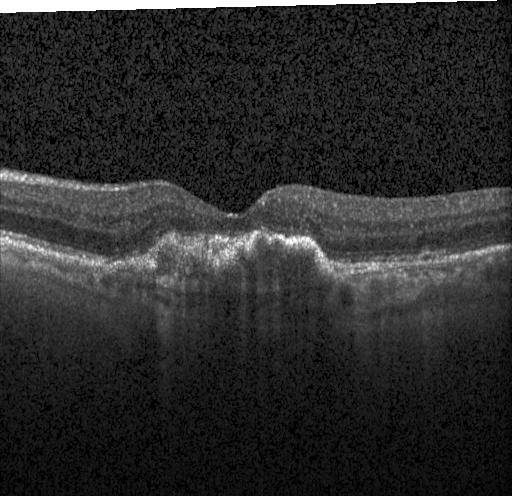
OCT line scan — Macular OCT: choroidal neovascularization (CNV).